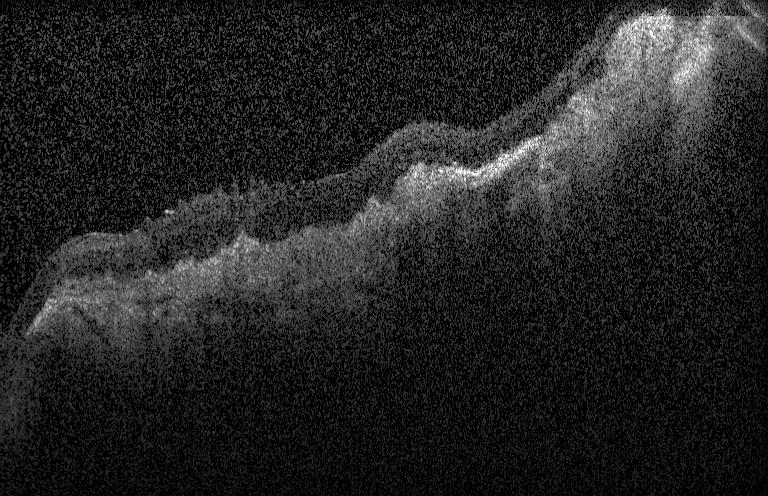 Diagnosis: CNV.